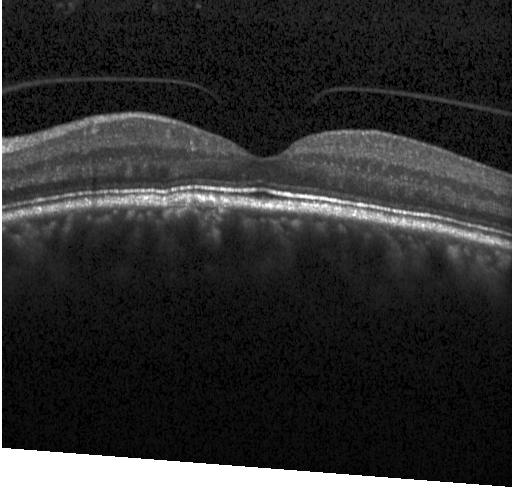
Dx: no choroidal neovascularization, diabetic macular edema, or drusen.